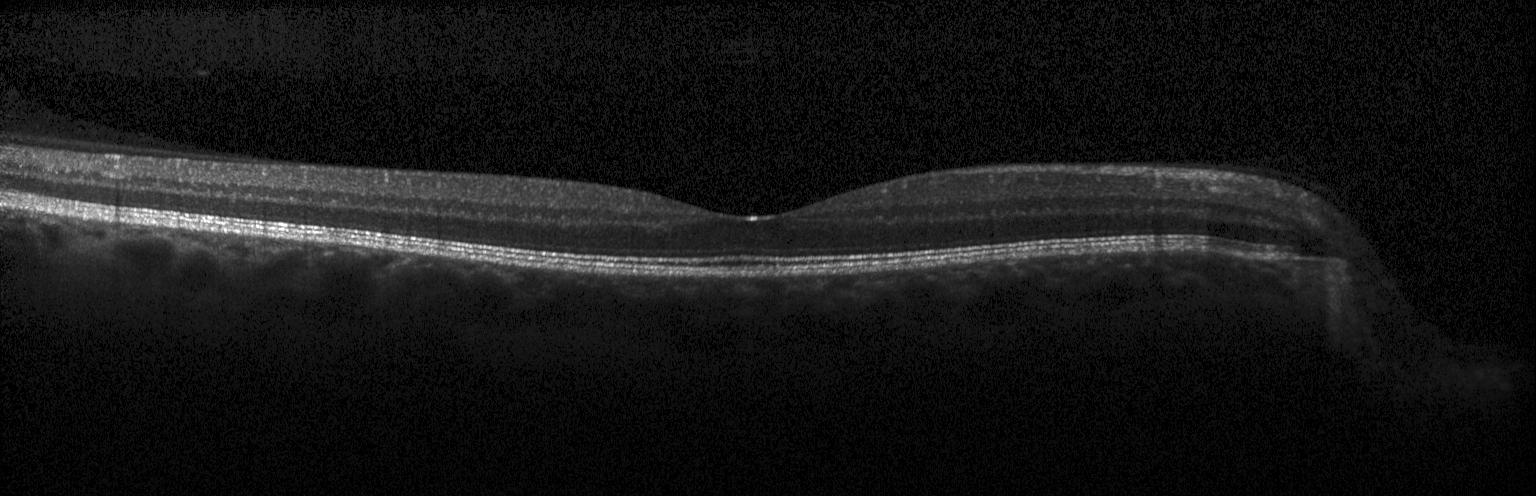 Optical coherence tomography B-scan. Dx: no evidence of choroidal neovascularization, diabetic macular edema, or drusen.